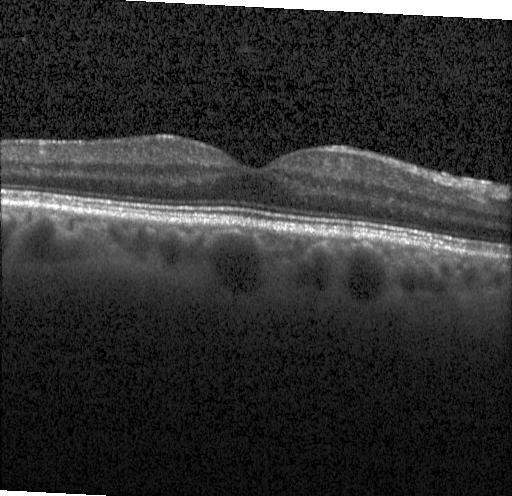
Optical coherence tomography B-scan
No choroidal neovascularization, no diabetic macular edema, and no drusen.